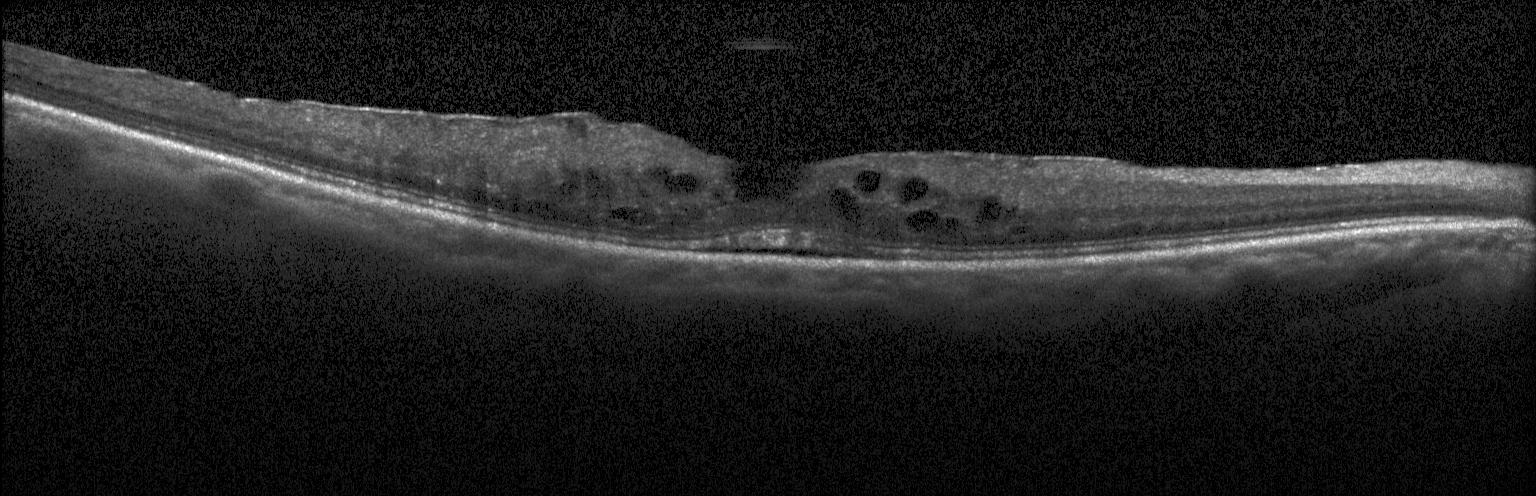 Spectral-domain OCT B-scan: DME.